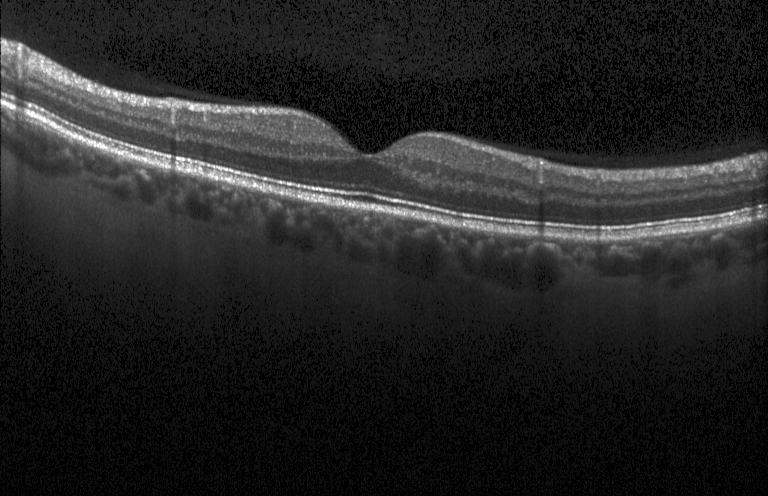 SD-OCT, horizontal scan through the fovea, Heidelberg Spectralis, OCT B-scan — Macular OCT: no evidence of choroidal neovascularization, diabetic macular edema, or drusen.